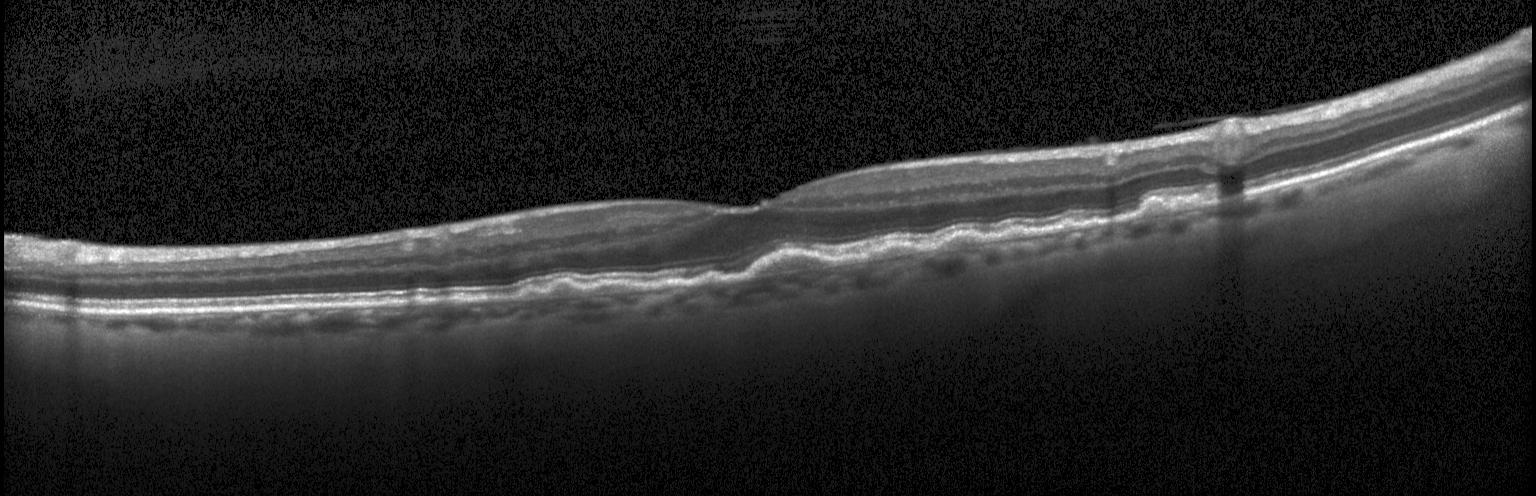

OCT finding: multiple drusen.